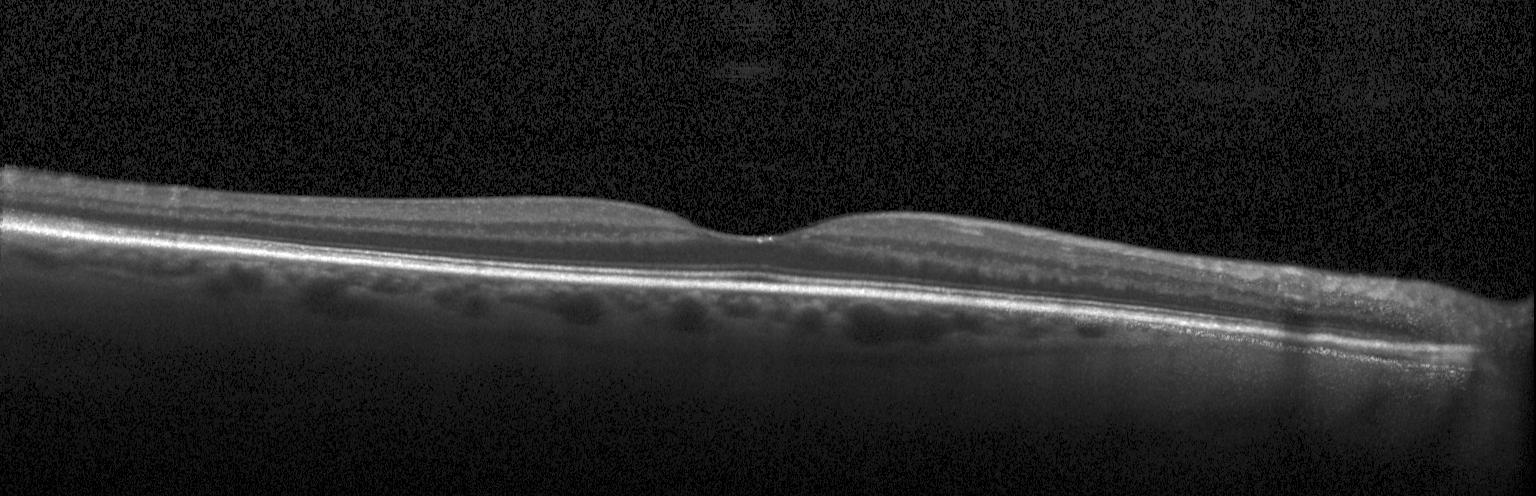
Optical coherence tomography B-scan. Heidelberg Spectralis OCT system — This B-scan demonstrates no choroidal neovascularization, no diabetic macular edema, and no drusen.